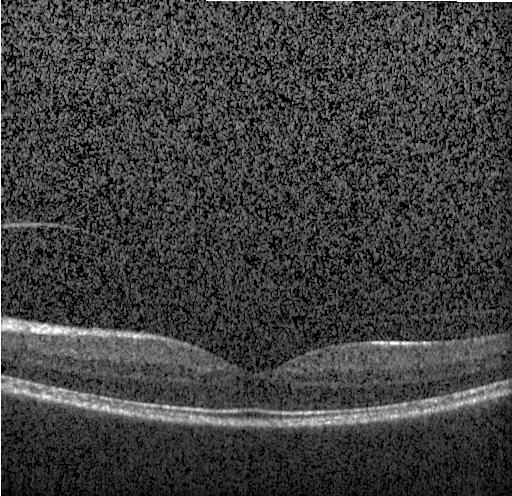 Spectral-domain OCT B-scan: no evidence of choroidal neovascularization, diabetic macular edema, or drusen.